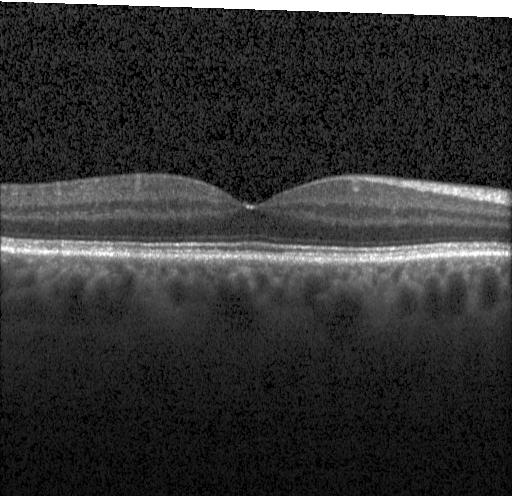 No choroidal neovascularization, no diabetic macular edema, and no drusen.